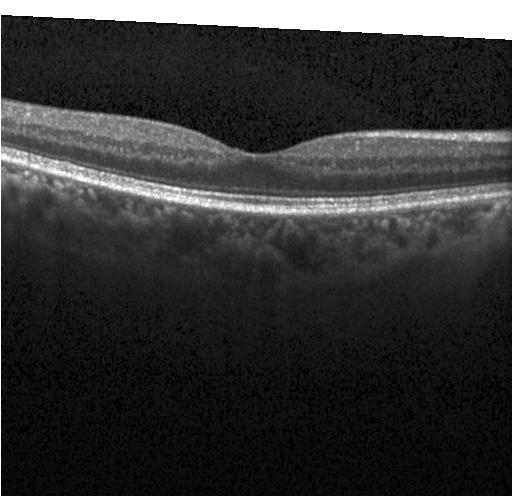
Macular OCT: neither choroidal neovascularization, diabetic macular edema, nor drusen.